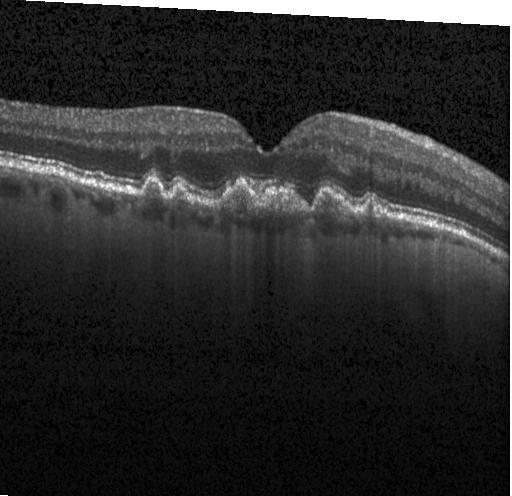

Optical coherence tomography B-scan — Finding: sub-RPE drusenoid deposits.